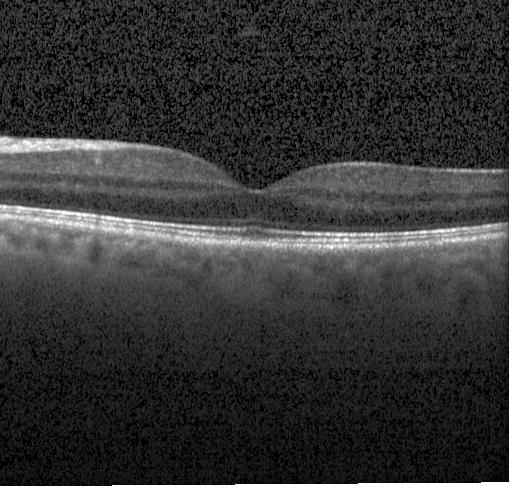 Diagnosis: neither CNV, DME, nor drusen.